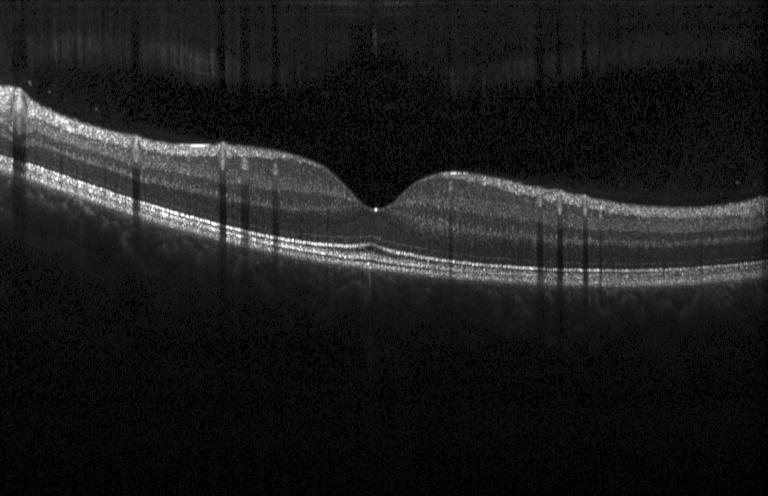

Acquired on a Heidelberg Spectralis, SD-OCT, optical coherence tomography scan — Dx: no choroidal neovascularization, diabetic macular edema, or drusen.